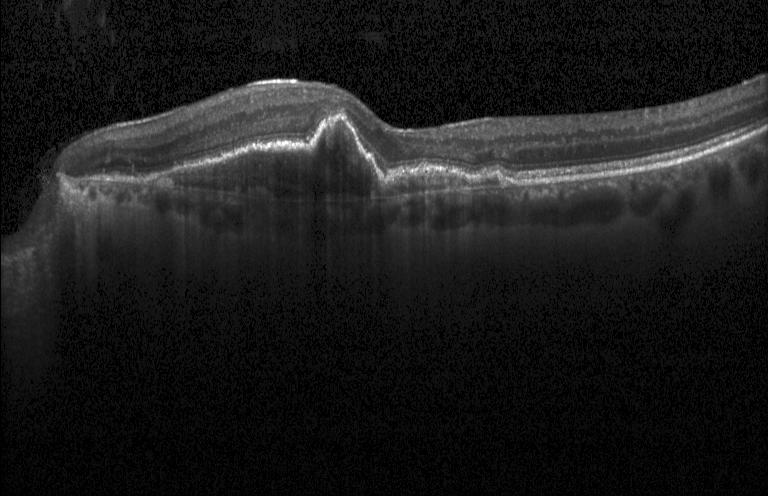

Macular scan. OCT line scan. Instrument: Heidelberg Spectralis. SD-OCT
Assessment: choroidal neovascularization (CNV).